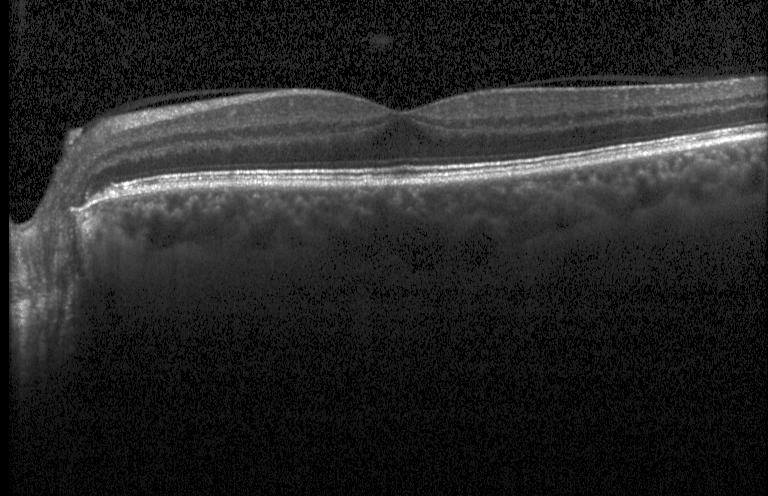

Spectral-domain optical coherence tomography, Heidelberg Spectralis, fovea-centered, OCT B-scan. Assessment: no evidence of choroidal neovascularization, diabetic macular edema, or drusen.